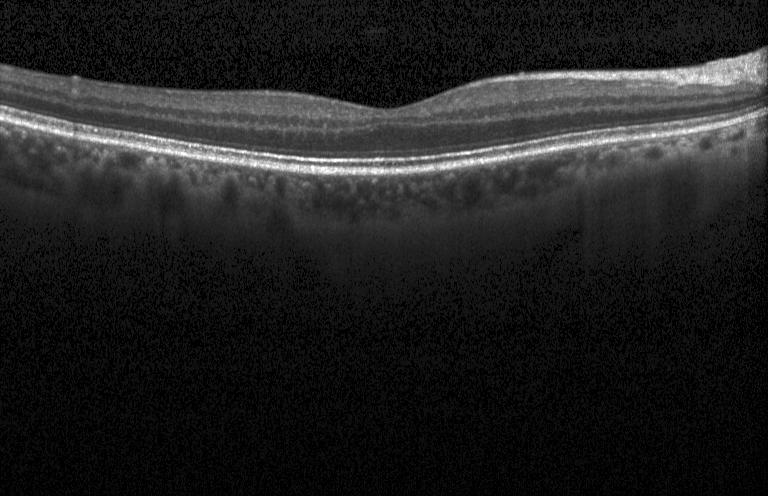 Neither CNV, DME, nor drusen.